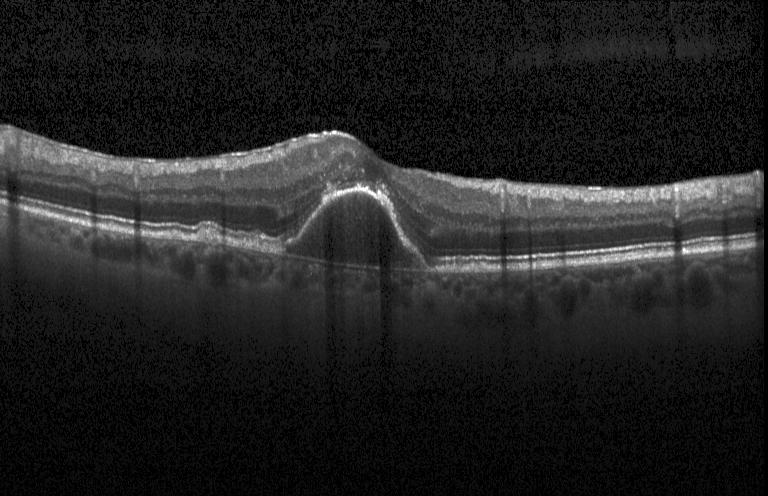 Retinal OCT cross-section showing choroidal neovascularization (CNV).